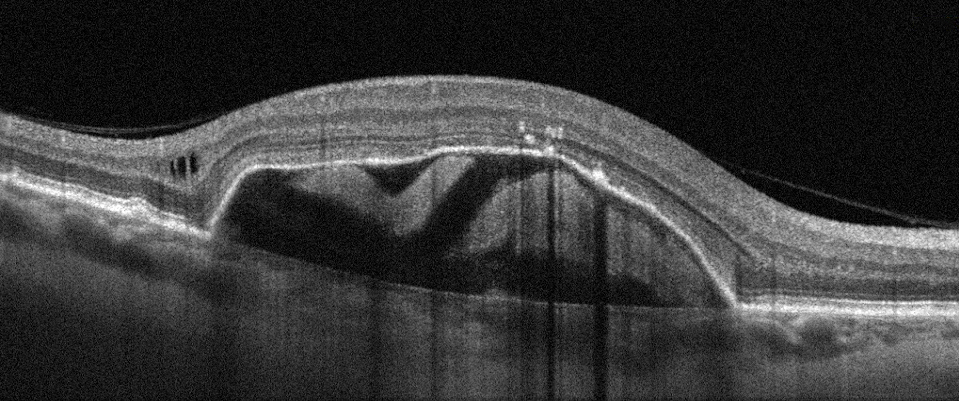 Macular OCT: AMD.